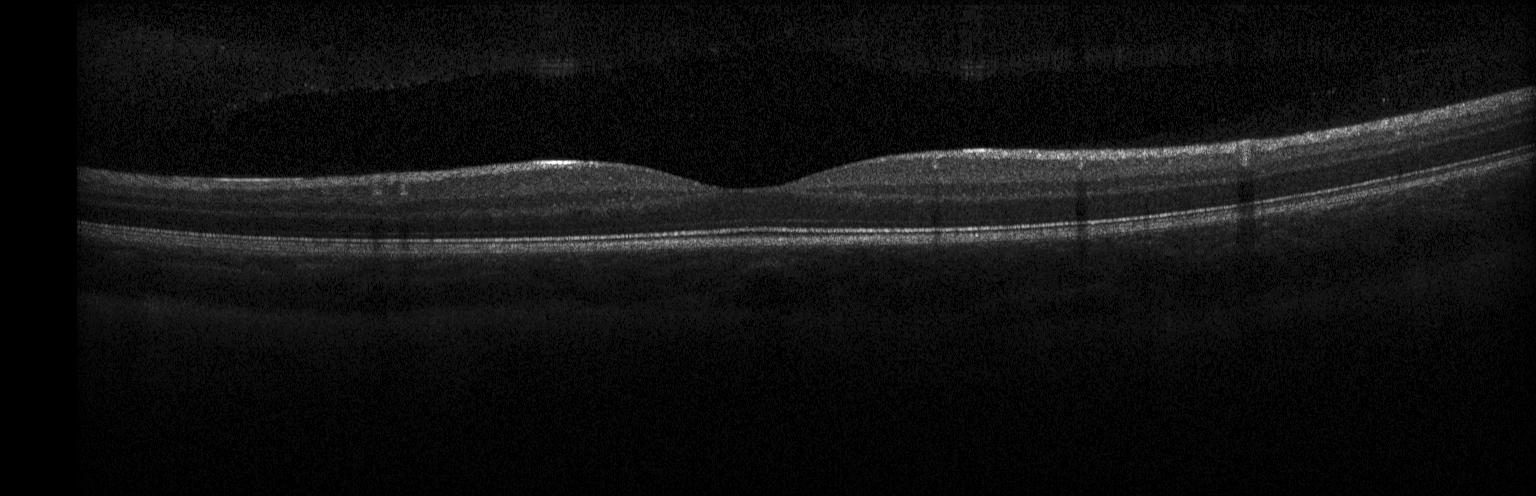

Optical coherence tomography B-scan. Diagnosis: neither choroidal neovascularization, diabetic macular edema, nor drusen.